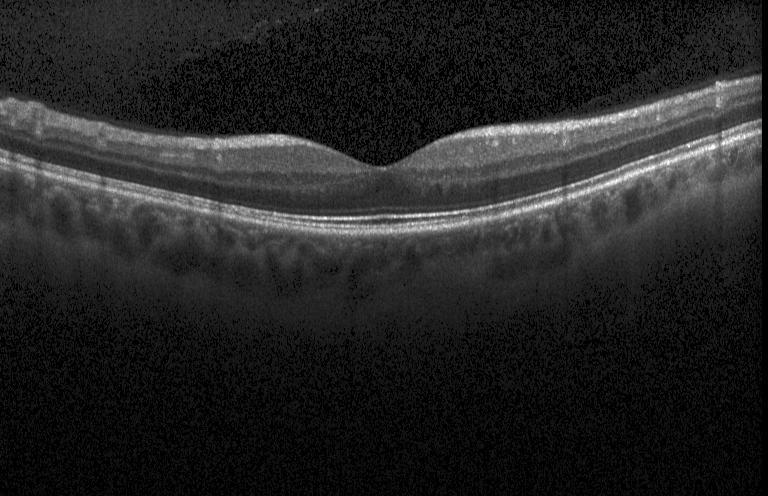 Optical coherence tomography B-scan · fovea-centered · SD-OCT · instrument: Heidelberg Spectralis
Impression: neither choroidal neovascularization, diabetic macular edema, nor drusen.